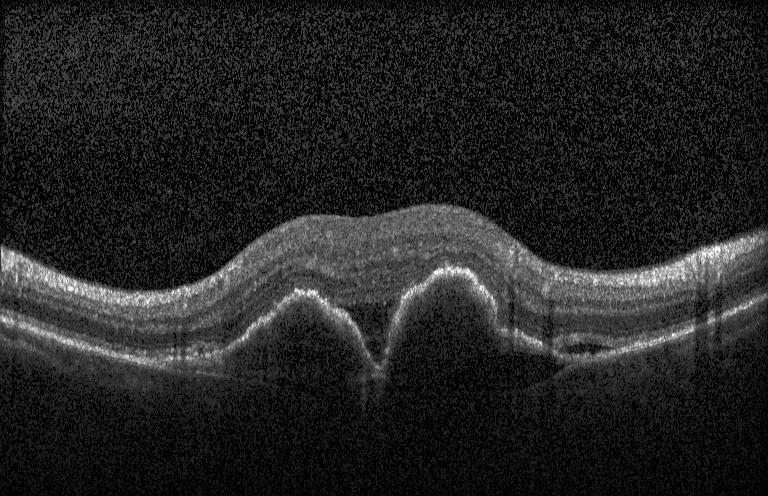

SD-OCT, optical coherence tomography B-scan, acquired on a Heidelberg Spectralis. Finding: choroidal neovascularization (CNV).